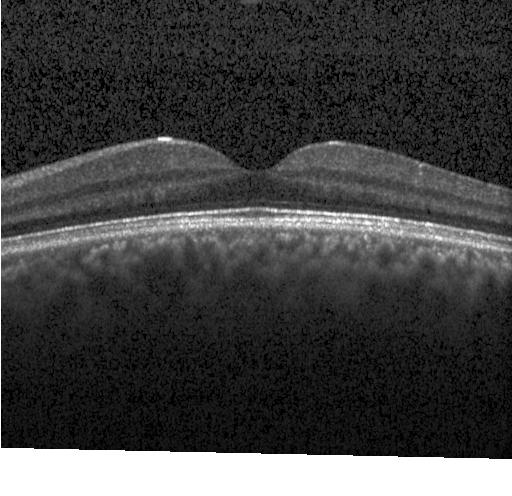

OCT B-scan. Diagnosis: neither choroidal neovascularization, diabetic macular edema, nor drusen.